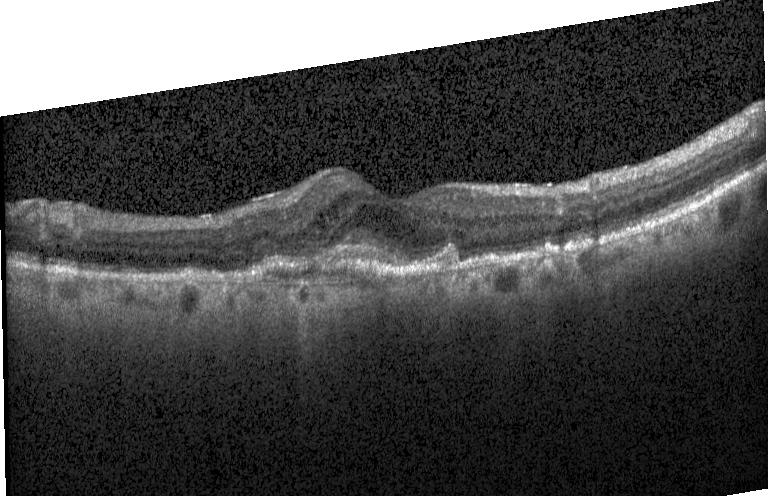

Finding: choroidal neovascularization.